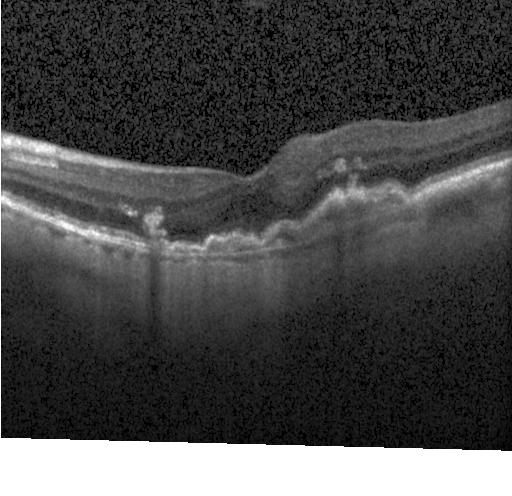 Optical coherence tomography scan.
Diagnosis: a choroidal neovascular membrane.